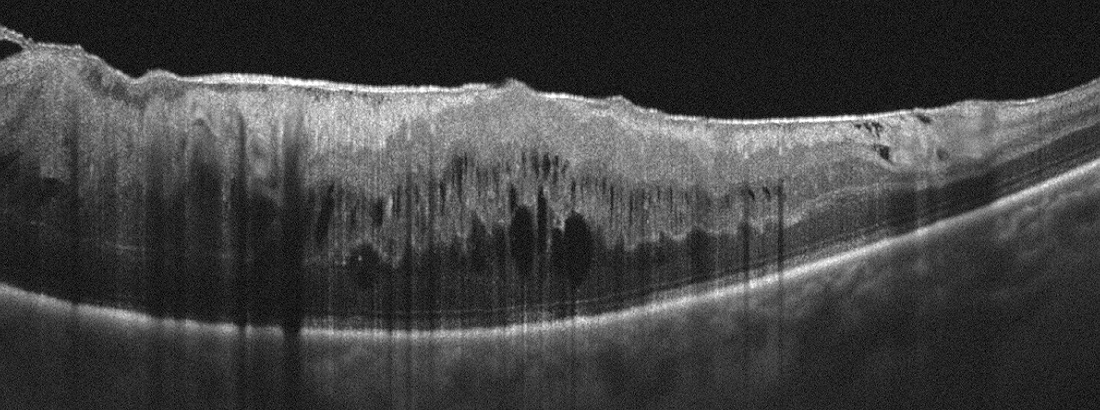

OCT scan showing ERM.